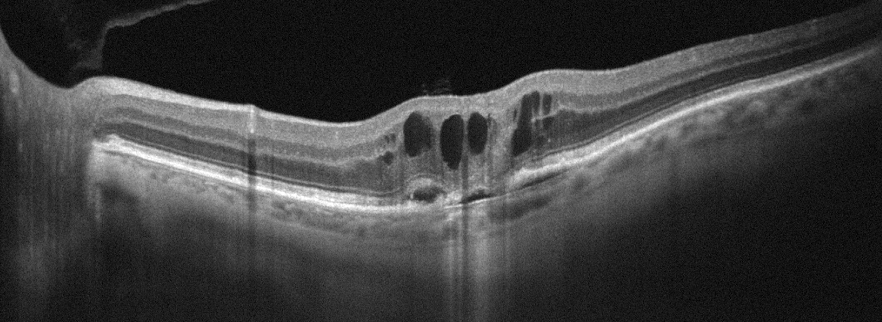 Acquired on an Optovue Avanti RTVue XR; macular scan; OCT line scan; OS.
Dx: AMD.